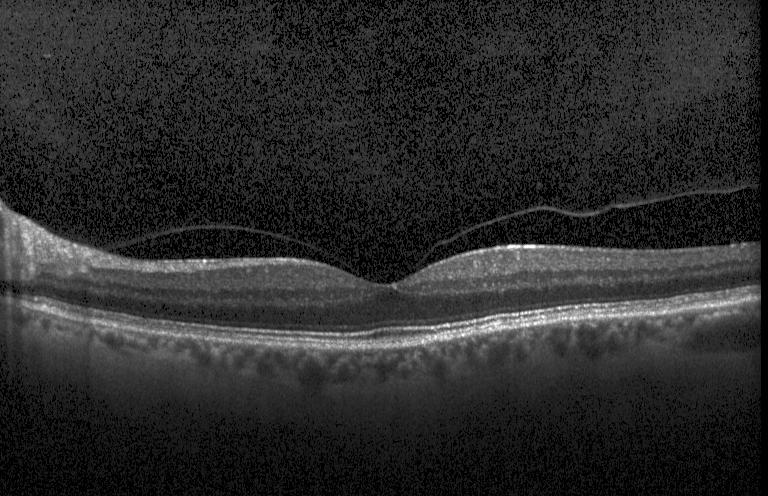

Spectral-domain OCT. Macular scan. OCT line scan. Heidelberg Spectralis
Diagnosis: no evidence of choroidal neovascularization, diabetic macular edema, or drusen.